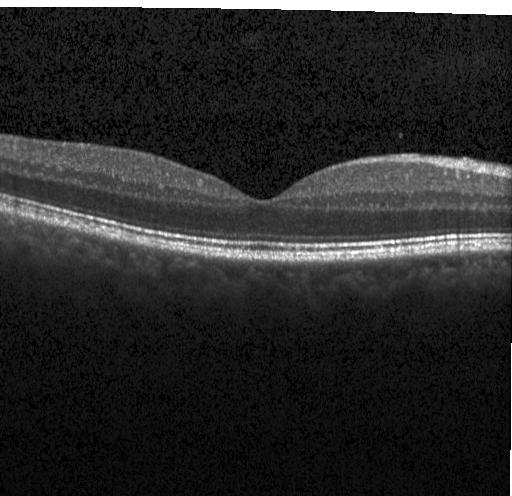 Optical coherence tomography scan. Heidelberg Spectralis OCT system
No CNV, DME, or drusen.